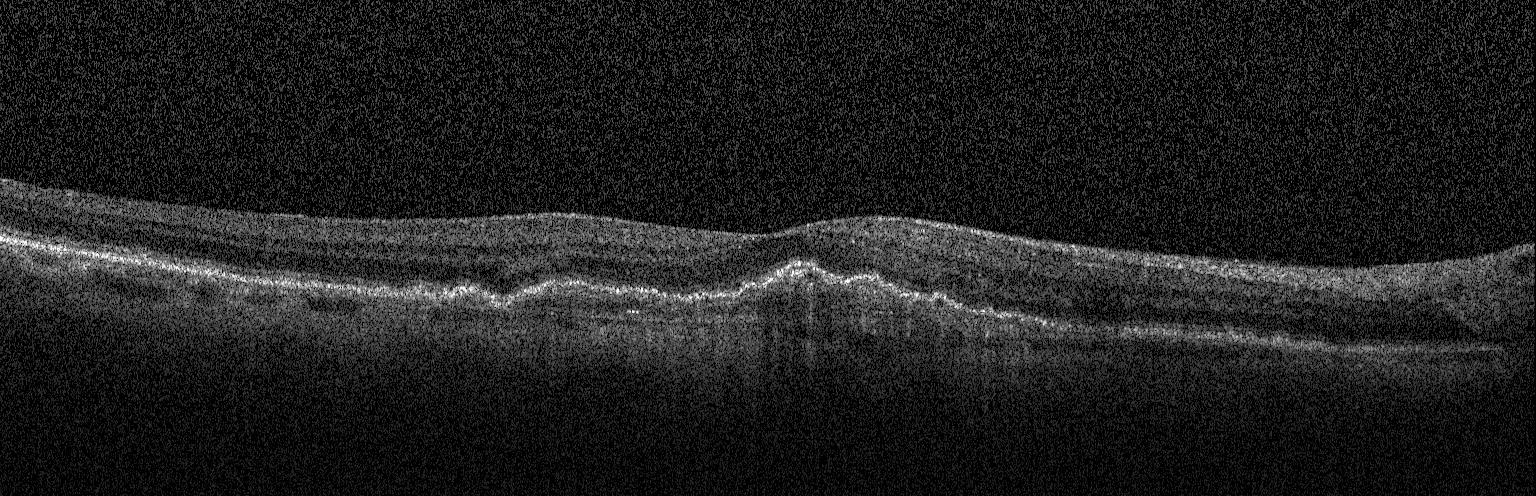 Spectral-domain OCT; Heidelberg Spectralis OCT system; OCT B-scan; horizontal scan through the fovea
Finding: a choroidal neovascular membrane.